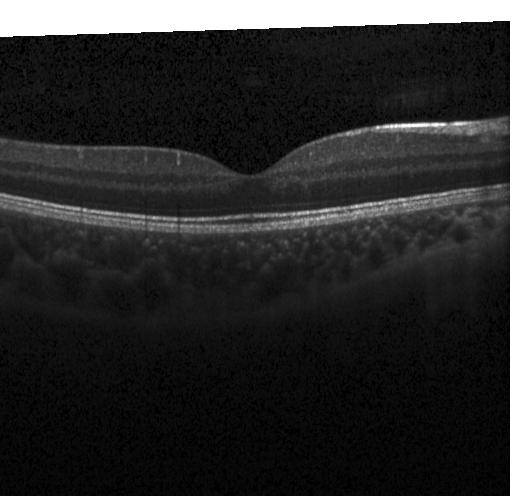

Spectral-domain OCT B-scan: no evidence of choroidal neovascularization, diabetic macular edema, or drusen.